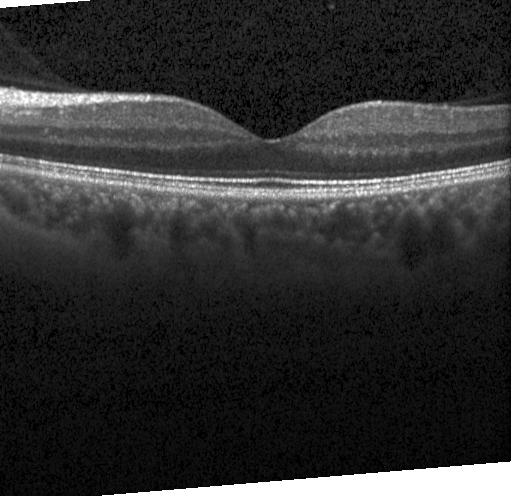
Diagnosis: no choroidal neovascularization, no diabetic macular edema, and no drusen.